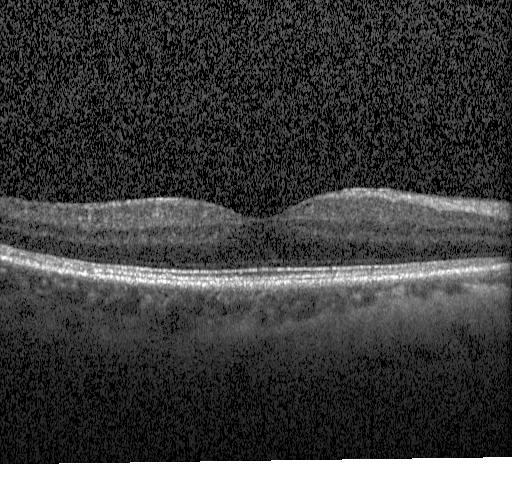

Macular OCT: no evidence of CNV, DME, or drusen.